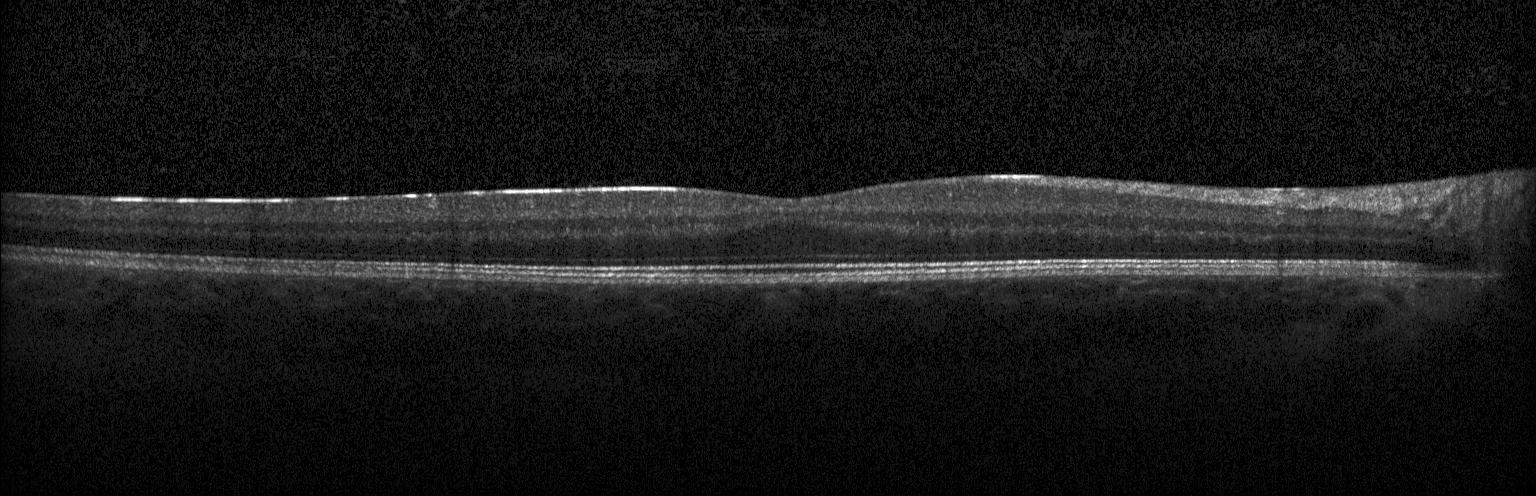

Acquired on a Heidelberg Spectralis, optical coherence tomography B-scan — Diagnosis: neither choroidal neovascularization, diabetic macular edema, nor drusen.